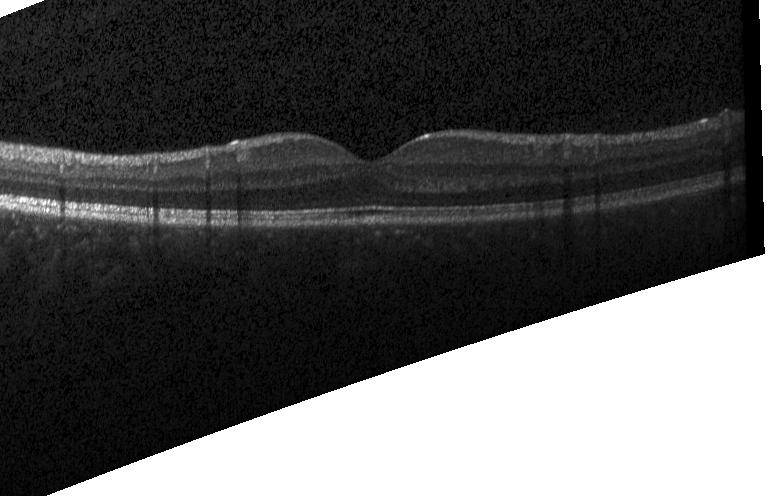

Impression: no evidence of choroidal neovascularization, diabetic macular edema, or drusen.